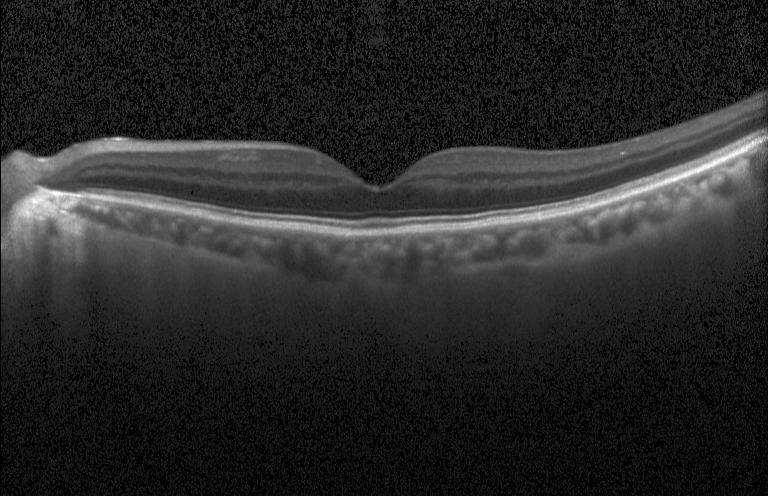
Spectral-domain OCT B-scan: no CNV, DME, or drusen.